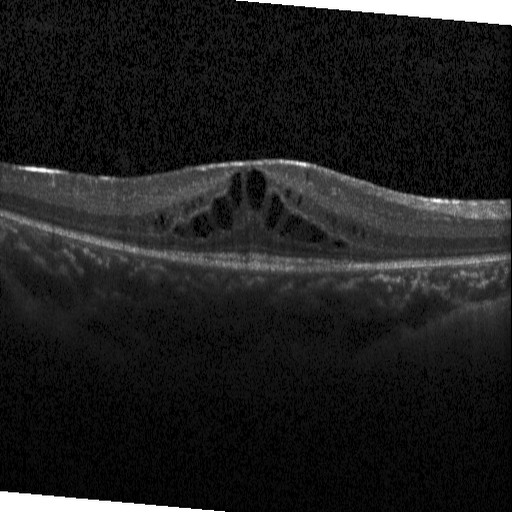 Retinal OCT cross-section · fovea-centered.
Macular OCT: diabetic macular edema.